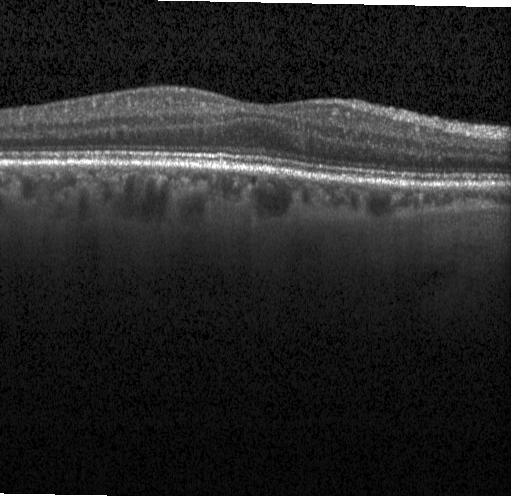
Fovea-centered, acquired on a Heidelberg Spectralis, SD-OCT, retinal OCT B-scan — Diagnosis: no choroidal neovascularization, no diabetic macular edema, and no drusen.